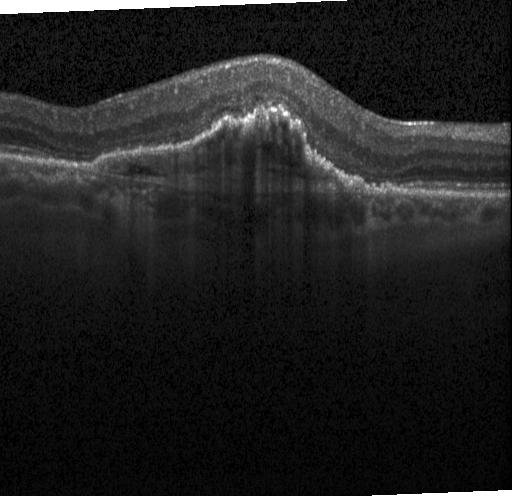 Instrument: Heidelberg Spectralis · SD-OCT · retinal OCT cross-section · through the macula — Finding: a choroidal neovascular membrane.